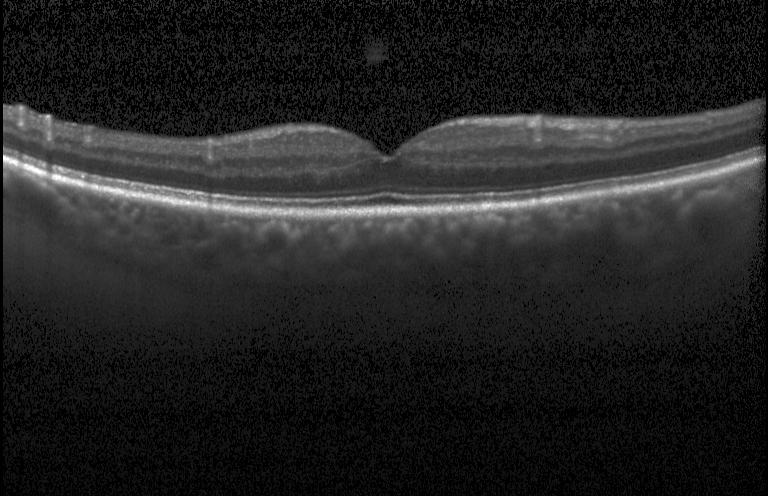
Heidelberg Spectralis; OCT B-scan; through the macula
Dx: no CNV, DME, or drusen.